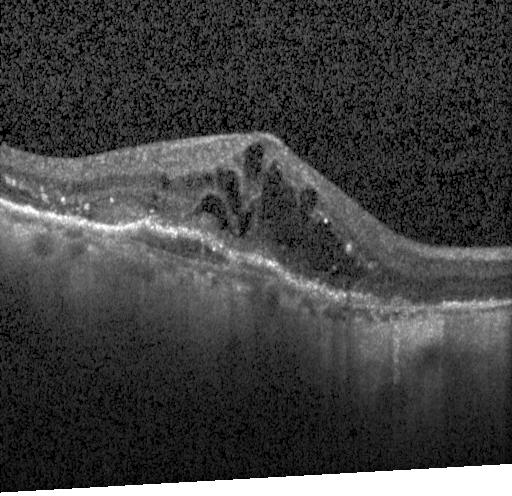

Impression: CNV.